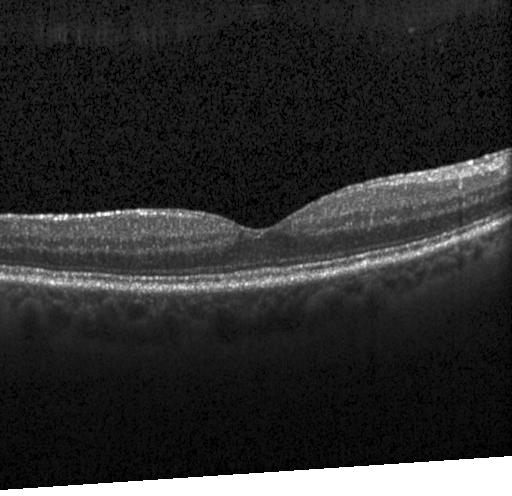 OCT B-scan showing neither choroidal neovascularization, diabetic macular edema, nor drusen.